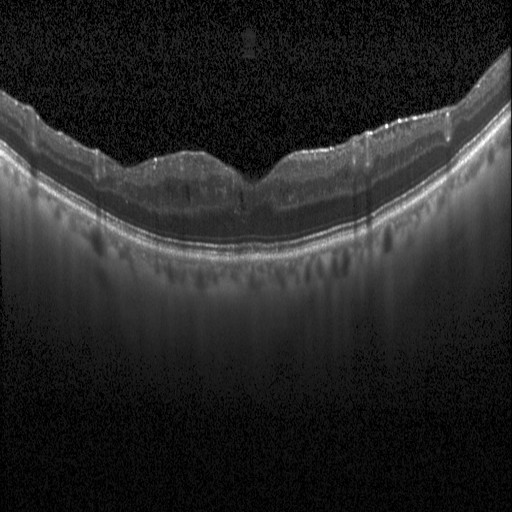

Heidelberg Spectralis, spectral-domain optical coherence tomography, retinal OCT cross-section — OCT finding: diabetic macular edema (DME).